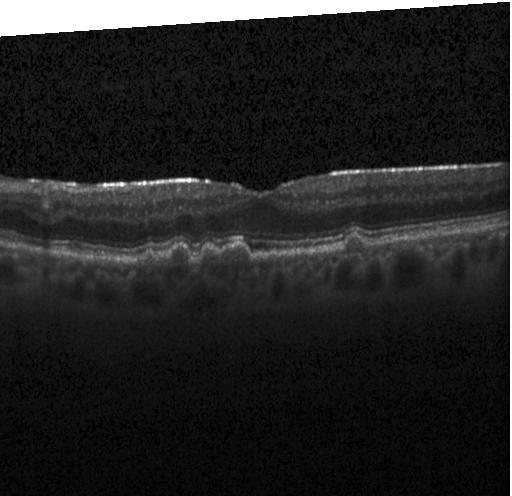 Optical coherence tomography B-scan. Impression: drusen.